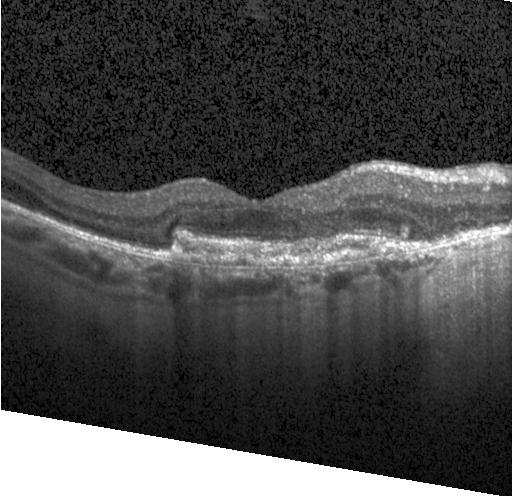
Diagnosis: CNV.